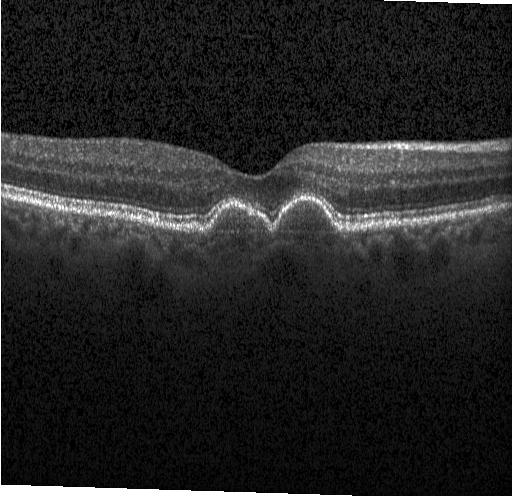
Acquired on a Heidelberg Spectralis, OCT line scan — Impression: multiple drusen.